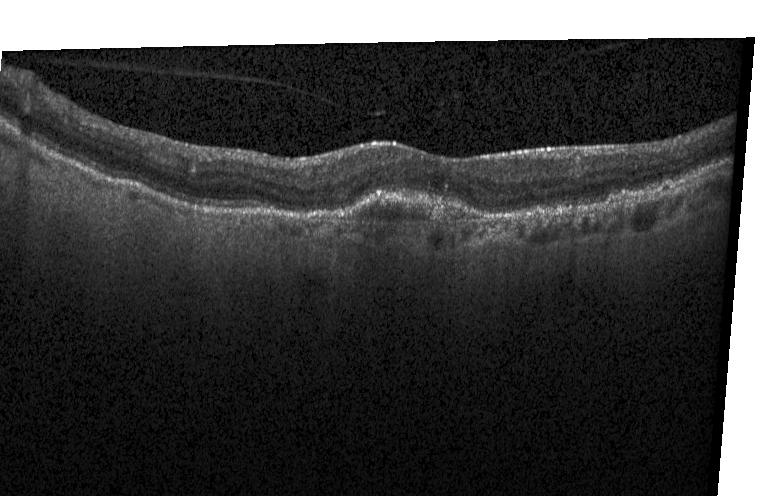

OCT line scan
This B-scan demonstrates a choroidal neovascular membrane.